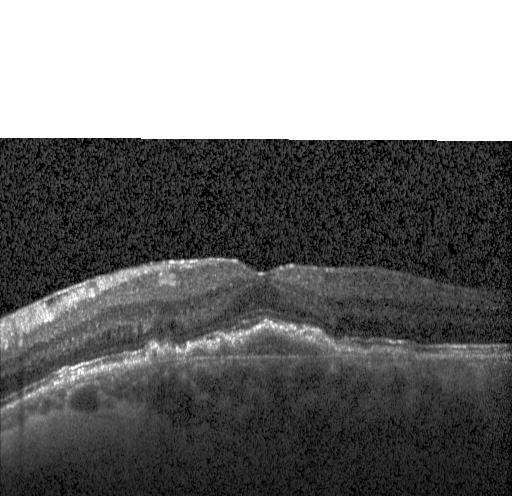

Heidelberg Spectralis, centered on the fovea, optical coherence tomography scan, SD-OCT
The scan shows a choroidal neovascular membrane.